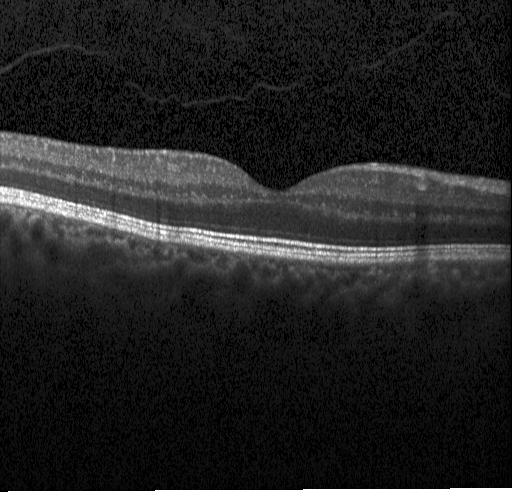 OCT line scan; acquired on a Heidelberg Spectralis; through the macula; spectral-domain OCT.
Macular OCT: no choroidal neovascularization, diabetic macular edema, or drusen.